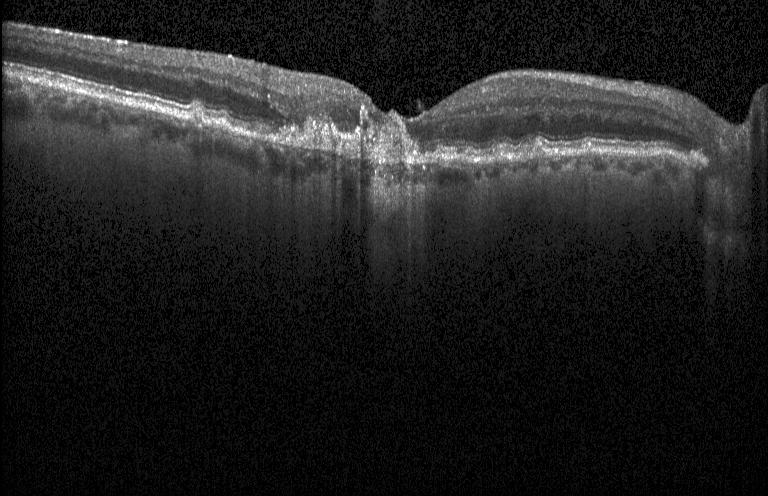

OCT line scan — Finding: a choroidal neovascular membrane.